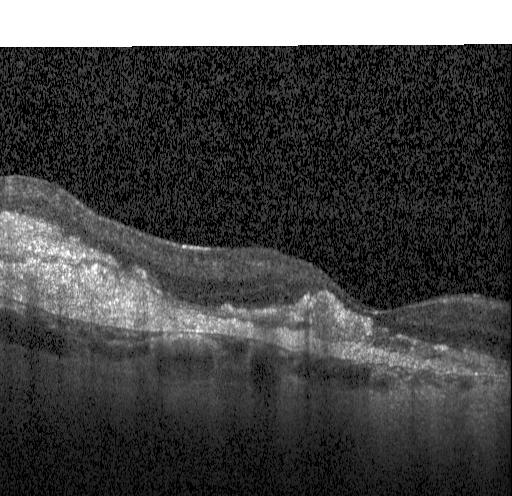

Fovea-centered. Spectral-domain optical coherence tomography. Retinal OCT B-scan
This B-scan demonstrates CNV.